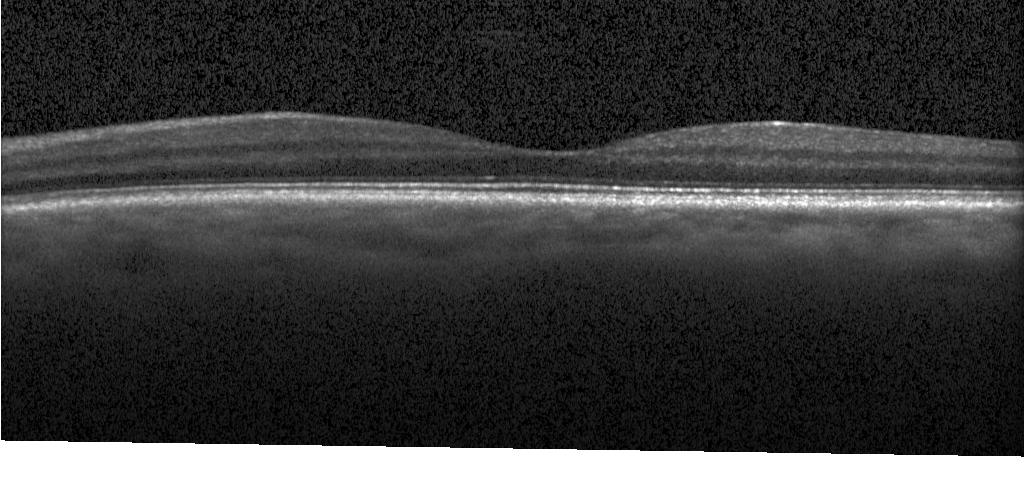 OCT B-scan showing no evidence of choroidal neovascularization, diabetic macular edema, or drusen.